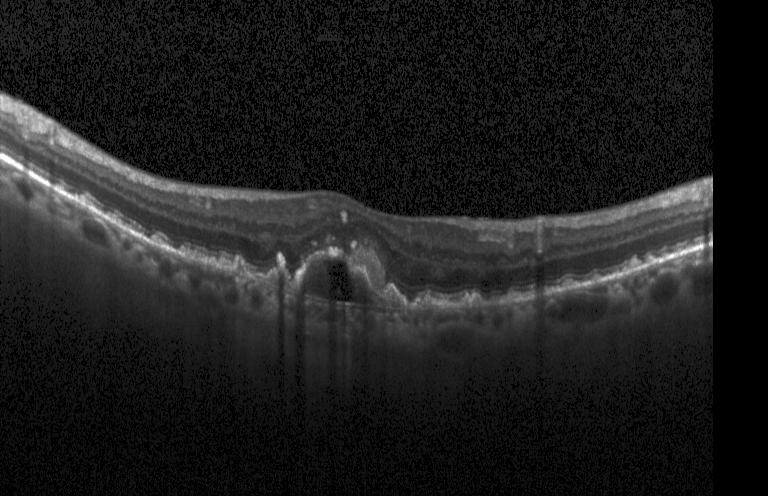

Optical coherence tomography B-scan — Finding: a choroidal neovascular membrane.